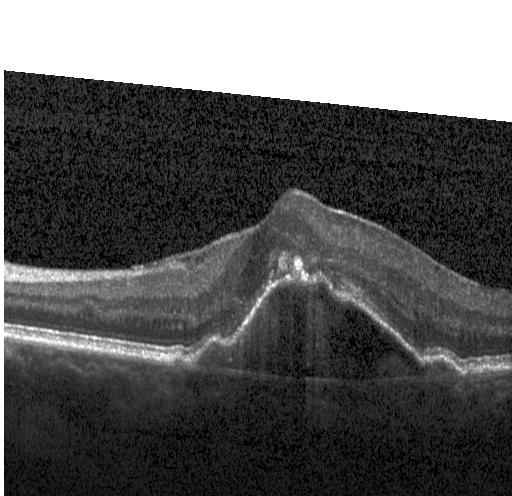 Fovea-centered · retinal OCT cross-section — A choroidal neovascular membrane.